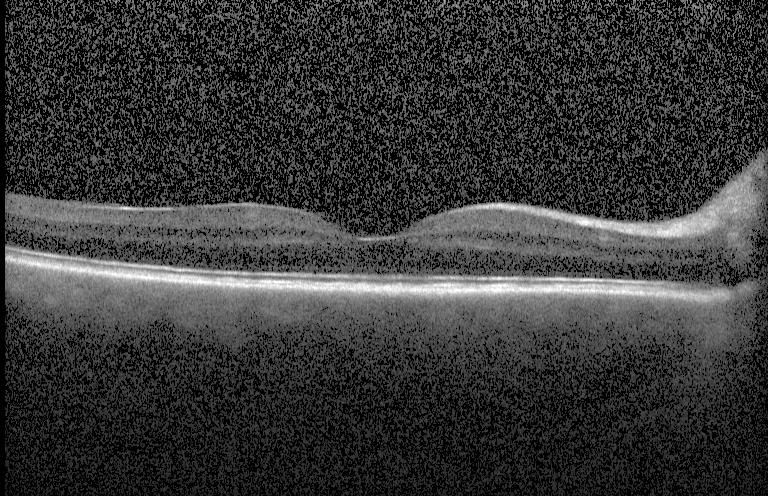
Macular OCT demonstrating neither CNV, DME, nor drusen.